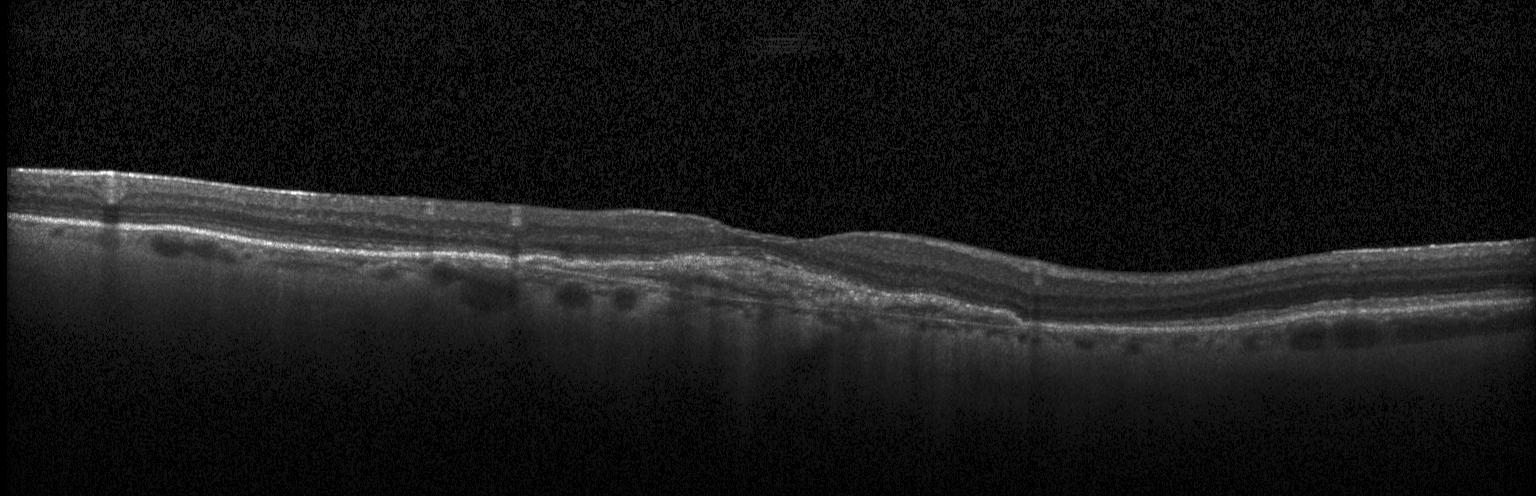 Finding: choroidal neovascularization (CNV).